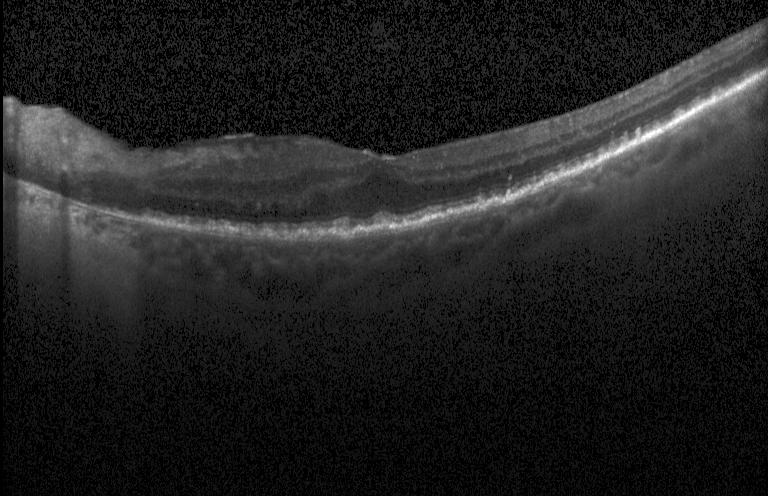
Heidelberg Spectralis OCT system; through the macula; optical coherence tomography B-scan — Diagnosis: drusen.